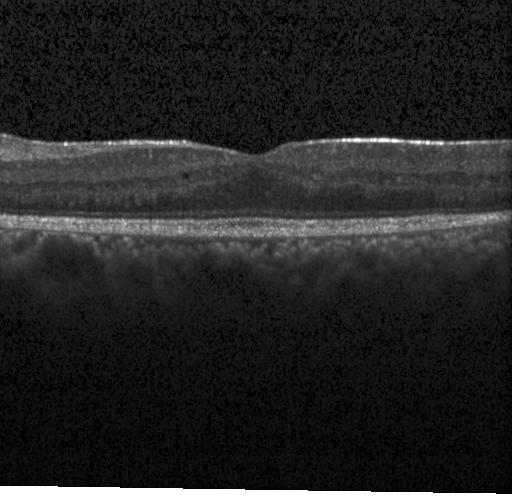
Dx: diabetic macular edema (DME).